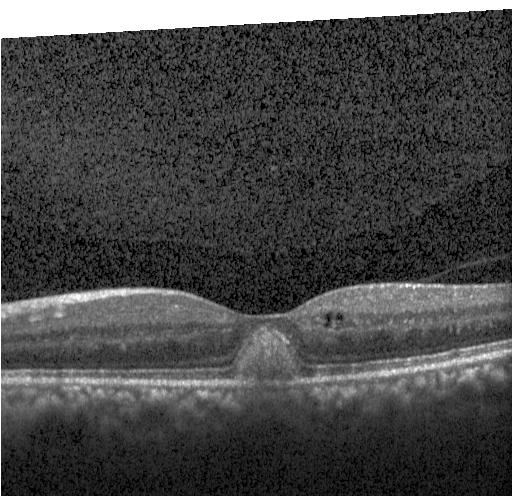

Macular scan, retinal OCT B-scan, SD-OCT — Macular OCT: a choroidal neovascular membrane.